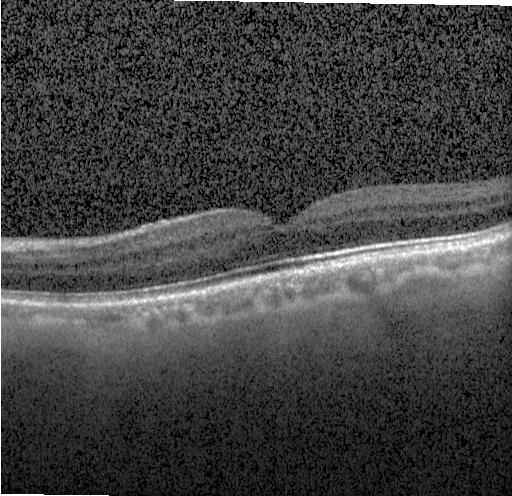 Through the macula, retinal OCT cross-section, acquired on a Heidelberg Spectralis.
Assessment: neither choroidal neovascularization, diabetic macular edema, nor drusen.